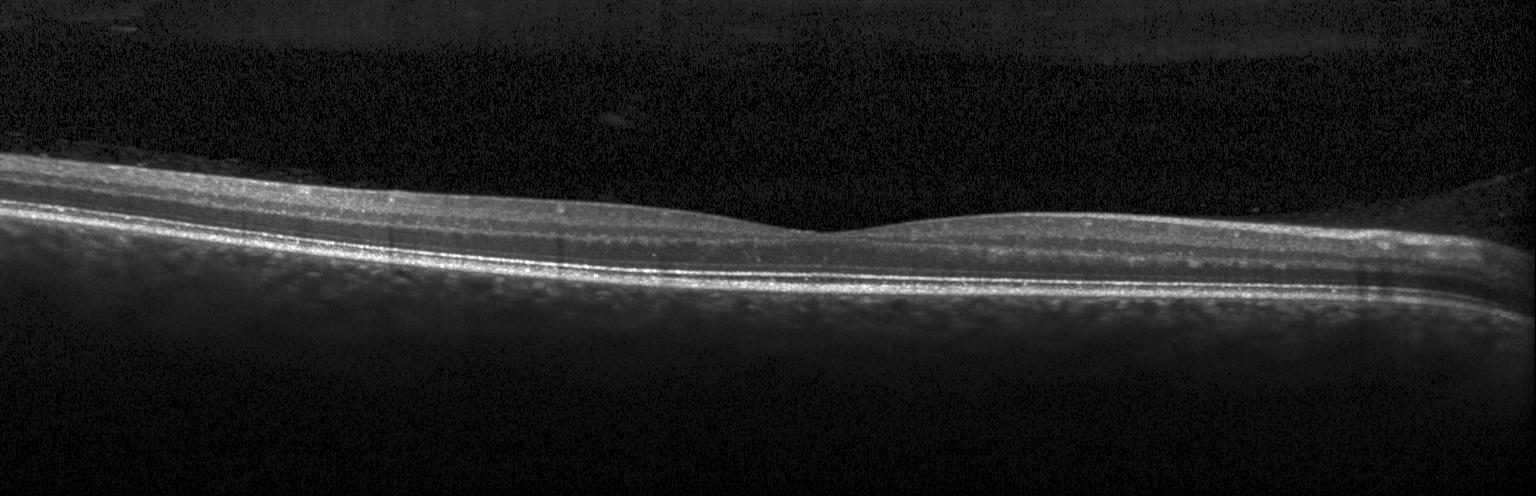
Horizontal scan through the fovea · spectral-domain optical coherence tomography · optical coherence tomography B-scan. Diagnosis: neither choroidal neovascularization, diabetic macular edema, nor drusen.